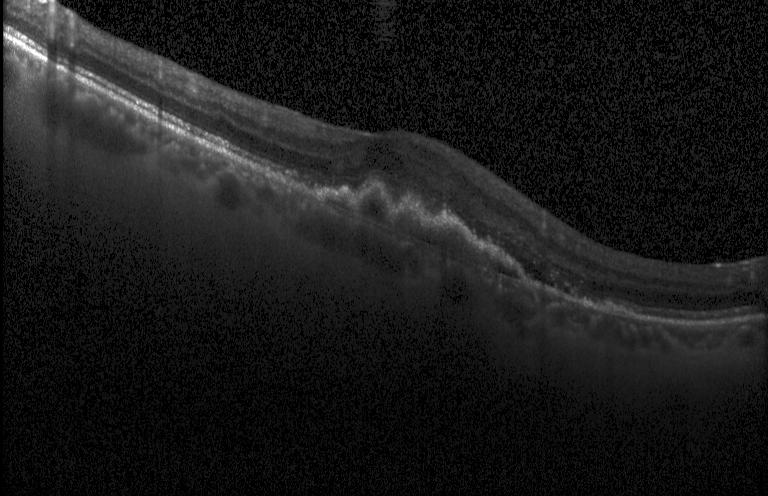 Diagnosis: a choroidal neovascular membrane.